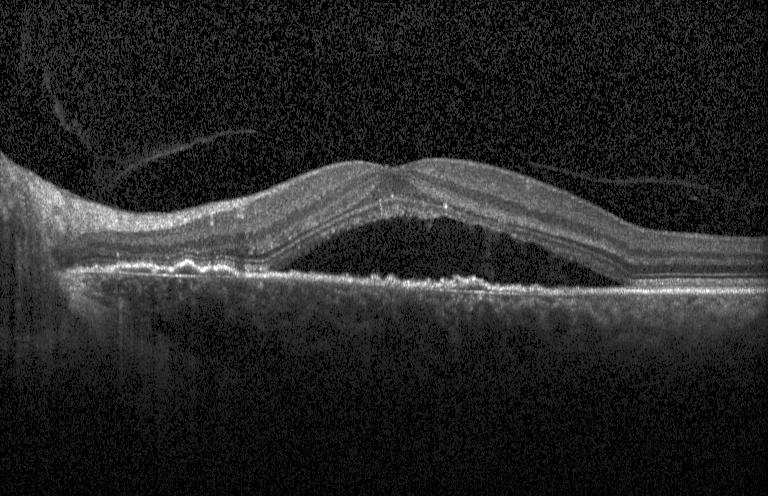

Macular OCT demonstrating a choroidal neovascular membrane.